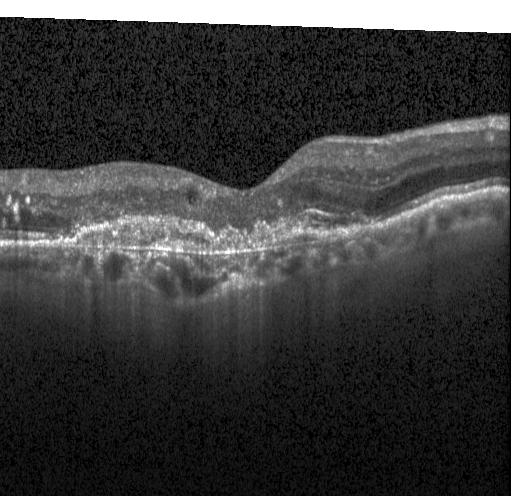 Horizontal scan through the fovea · retinal OCT cross-section — Impression: CNV.